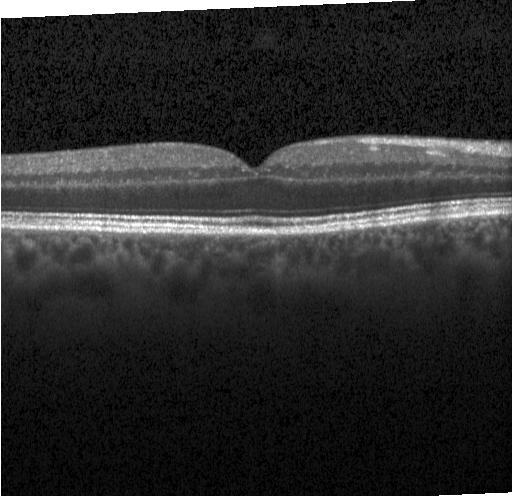 SD-OCT; Heidelberg Spectralis; optical coherence tomography scan — Finding: no evidence of choroidal neovascularization, diabetic macular edema, or drusen.